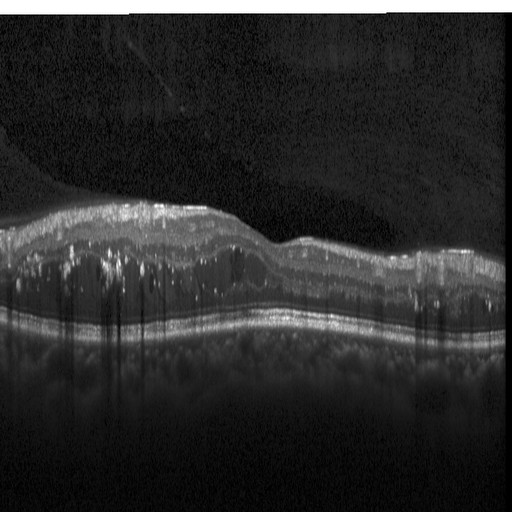
Fovea-centered · OCT B-scan
Macular OCT: diabetic macular edema (DME).